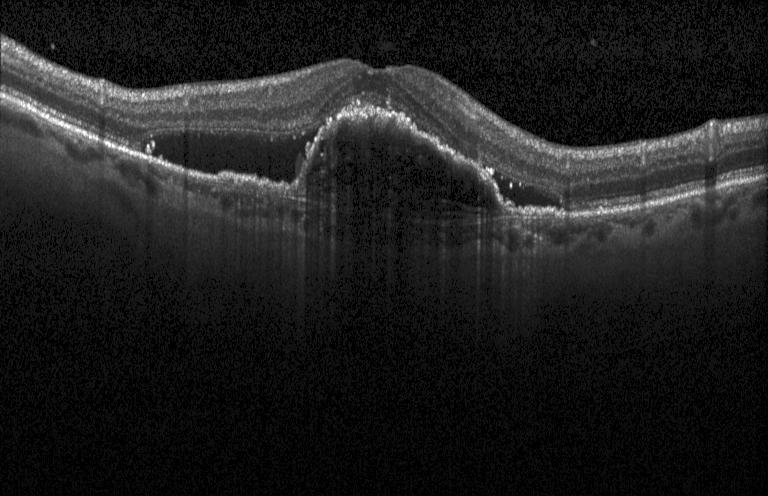 Optical coherence tomography scan — The scan shows CNV.